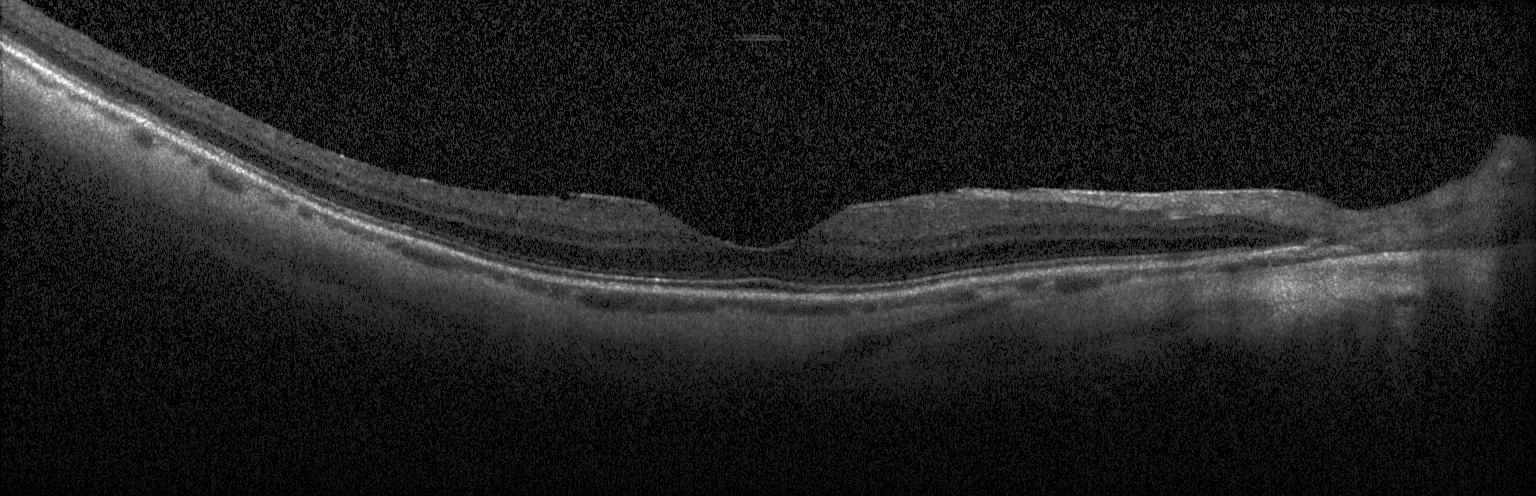 Neither choroidal neovascularization, diabetic macular edema, nor drusen.